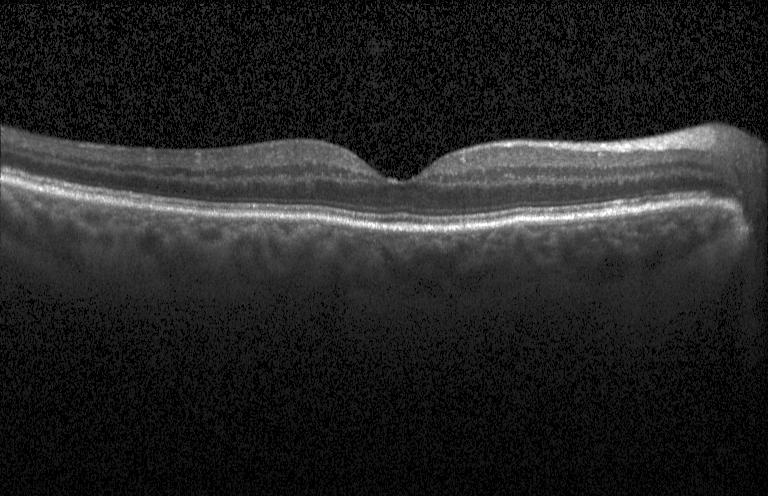

Retinal OCT cross-section
Impression: neither choroidal neovascularization, diabetic macular edema, nor drusen.